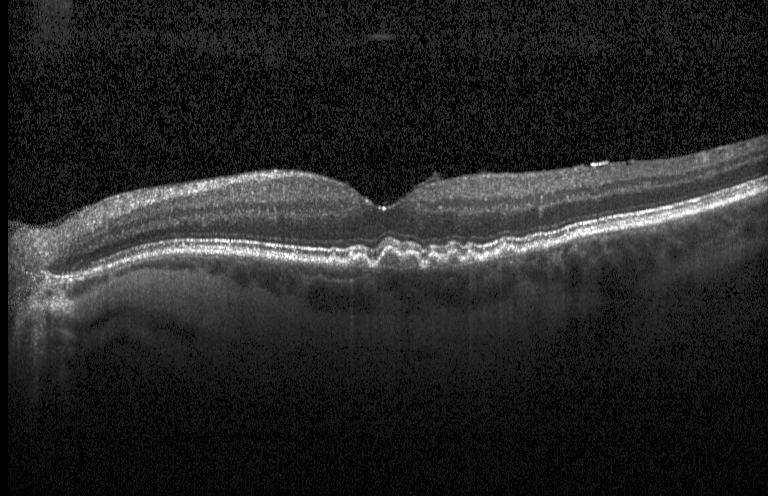
OCT scan showing multiple drusen.